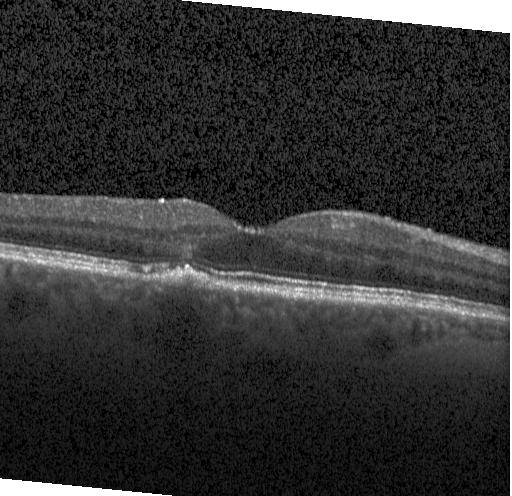

Optical coherence tomography scan — The scan shows sub-RPE drusenoid deposits.